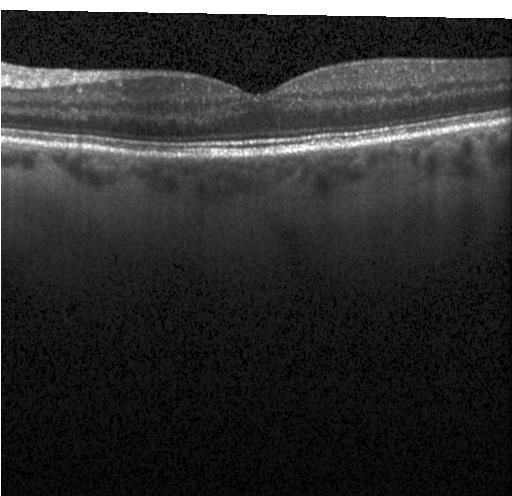 Diagnosis: no choroidal neovascularization, no diabetic macular edema, and no drusen.